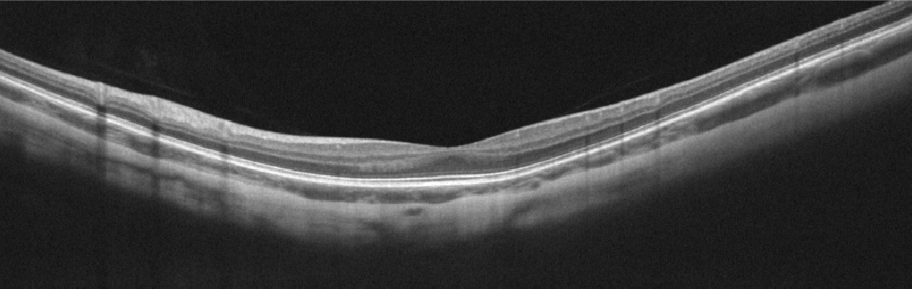 Optical coherence tomography scan — OCT finding: absence of AMD, DME, ERM, RAO, RVO, and vitreomacular interface disease.